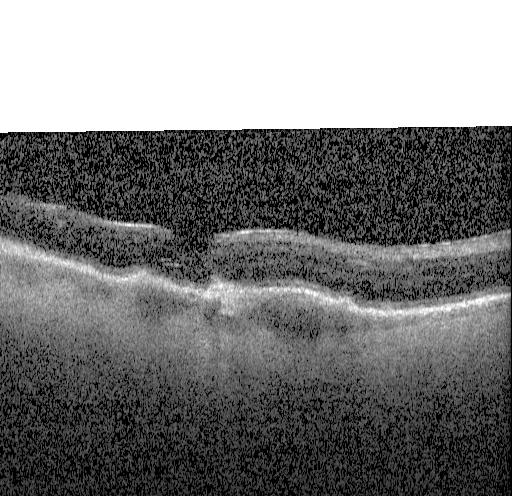 Retinal OCT B-scan — Impression: a choroidal neovascular membrane.